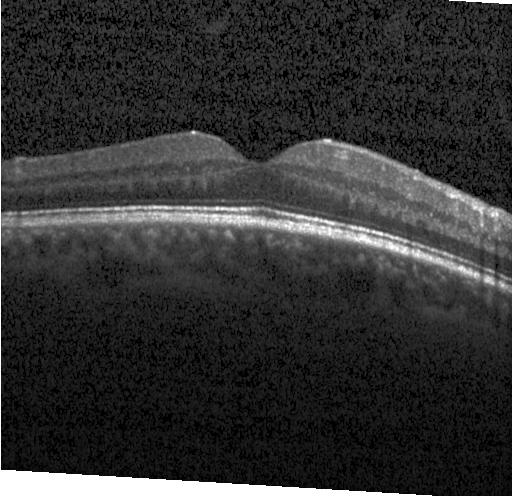

SD-OCT · optical coherence tomography B-scan · instrument: Heidelberg Spectralis · centered on the fovea — Diagnosis: neither CNV, DME, nor drusen.